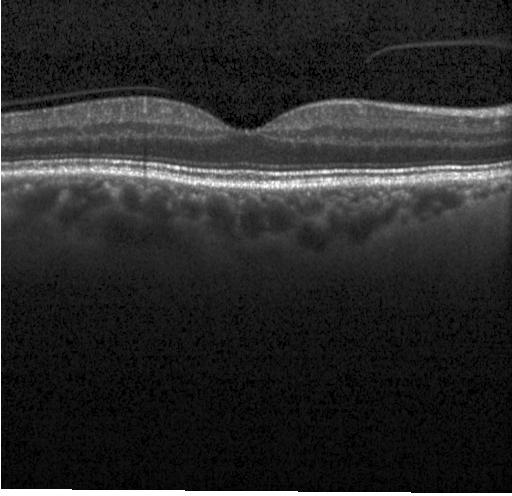

Retinal OCT cross-section.
This B-scan demonstrates no evidence of choroidal neovascularization, diabetic macular edema, or drusen.